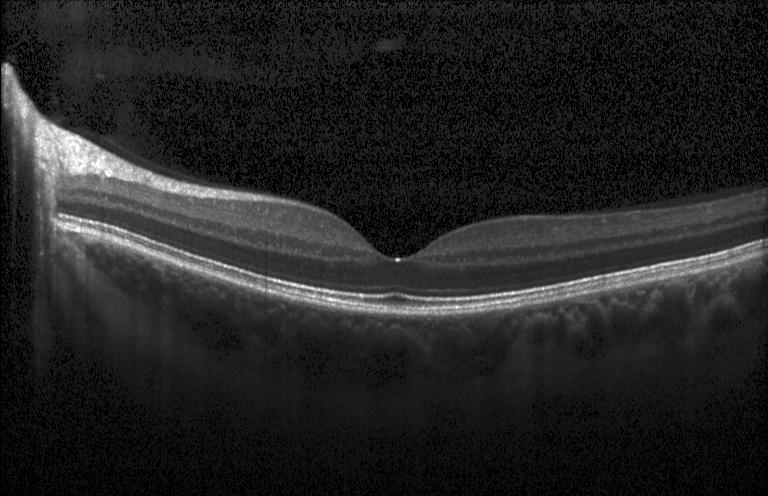

Assessment: no choroidal neovascularization, diabetic macular edema, or drusen.